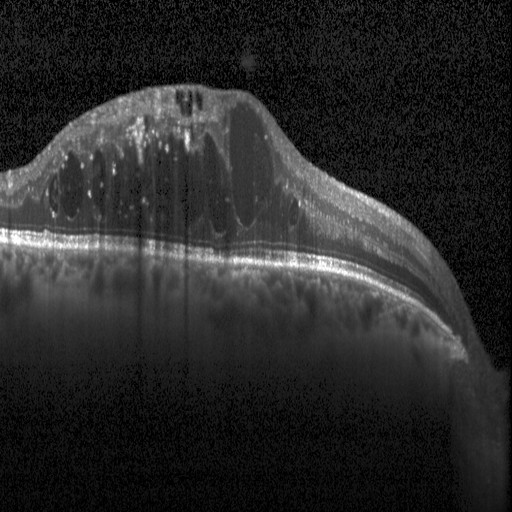

OCT finding: DME.